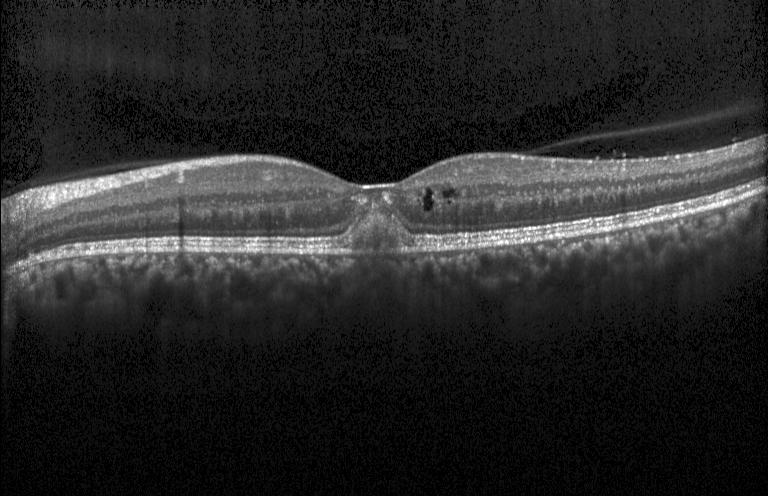
OCT B-scan showing a choroidal neovascular membrane.